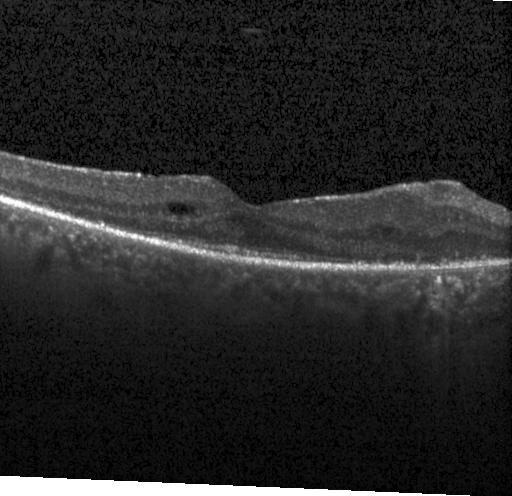

Retinal OCT B-scan — Diagnosis: diabetic macular edema (DME).